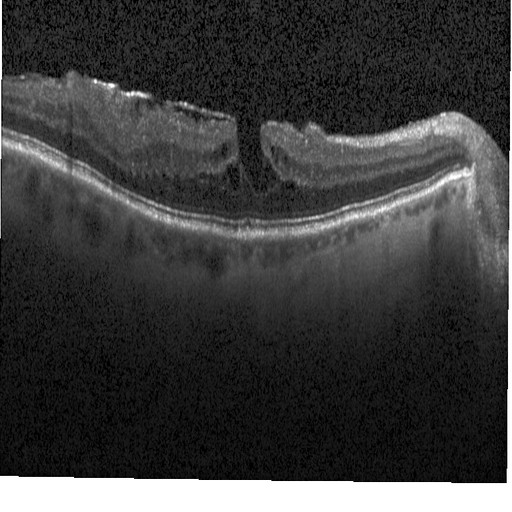 Horizontal scan through the fovea, Heidelberg Spectralis OCT system, OCT B-scan — Diabetic macular edema (DME).